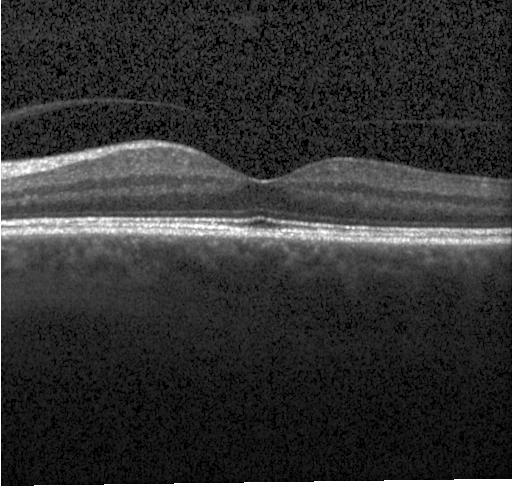
SD-OCT, optical coherence tomography scan, fovea-centered, Heidelberg Spectralis OCT system — OCT finding: no CNV, no DME, and no drusen.